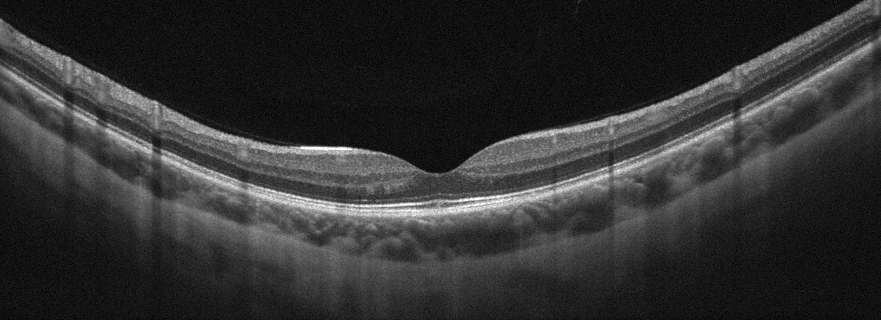 Left eye. Instrument: Optovue Avanti RTVue XR. Macular scan. OCT B-scan
Finding: no AMD, DME, ERM, RAO, RVO, or VID.